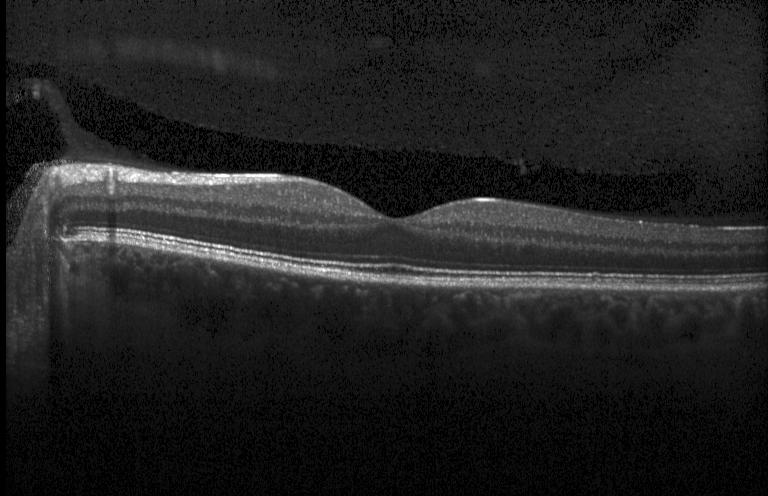 Spectral-domain optical coherence tomography. Optical coherence tomography B-scan — Diagnosis: no CNV, no DME, and no drusen.